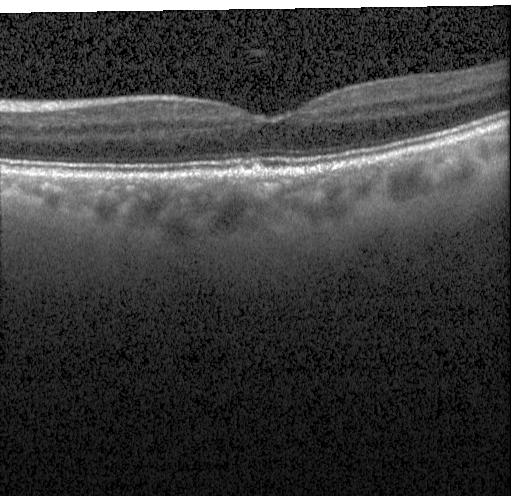 OCT line scan — Assessment: sub-RPE drusenoid deposits.